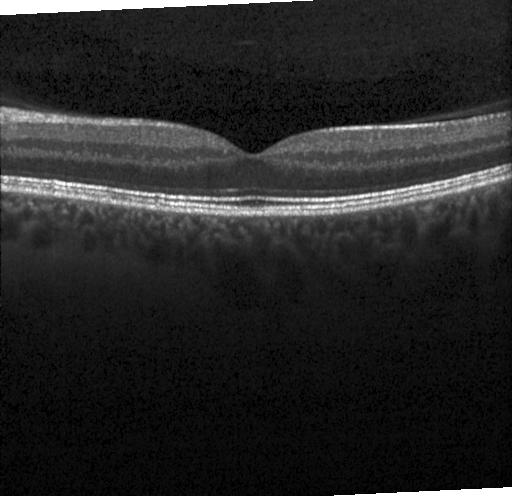

Optical coherence tomography B-scan. Instrument: Heidelberg Spectralis. SD-OCT. Horizontal scan through the fovea
Impression: no evidence of choroidal neovascularization, diabetic macular edema, or drusen.